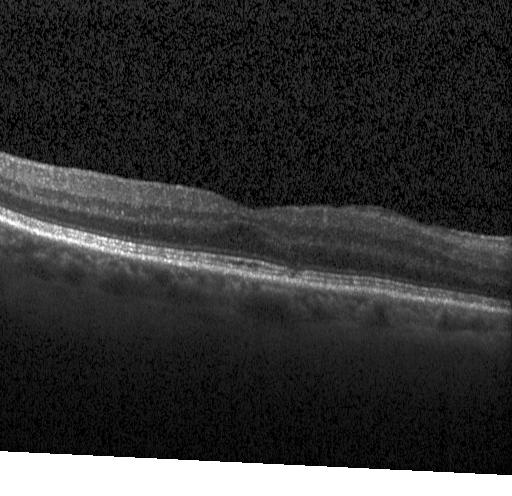
Horizontal scan through the fovea, retinal OCT B-scan — Finding: no evidence of choroidal neovascularization, diabetic macular edema, or drusen.